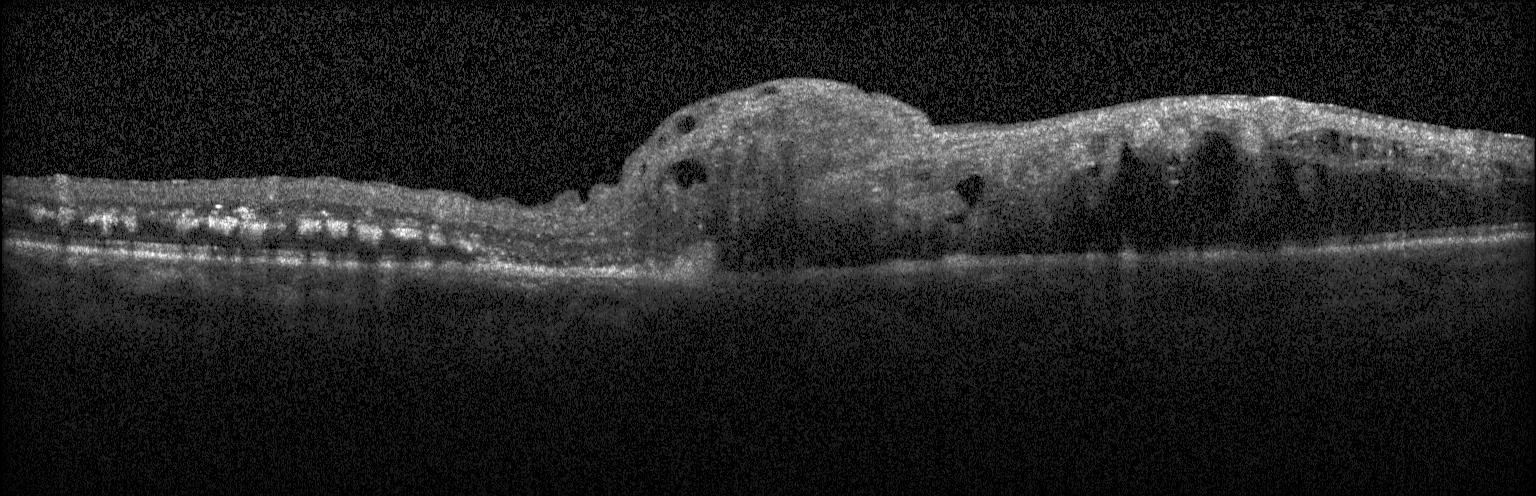 Finding: choroidal neovascularization.